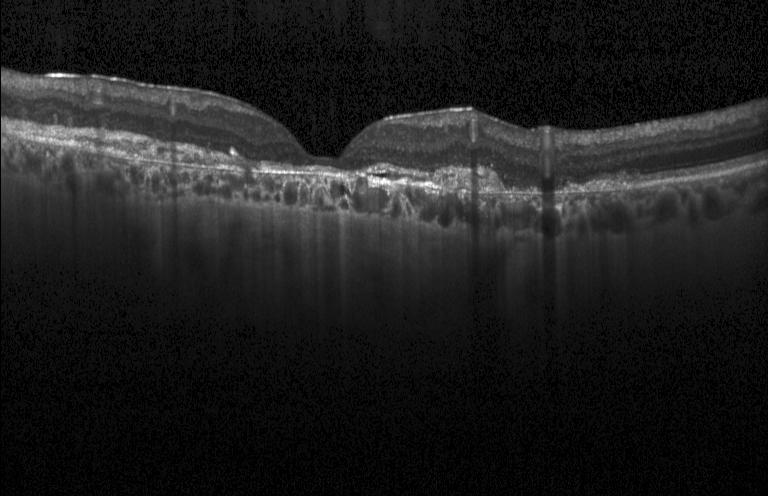
Impression: choroidal neovascularization.